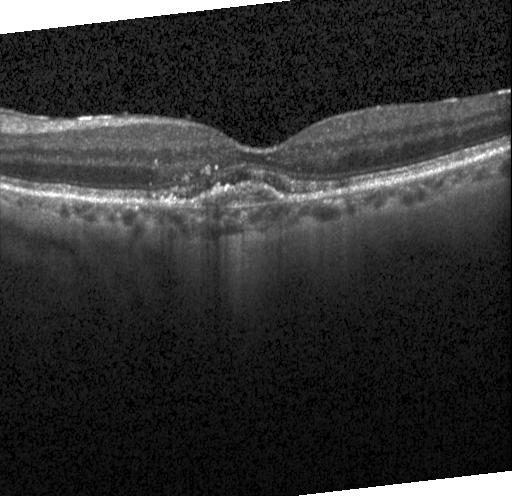 Centered on the fovea, SD-OCT, OCT B-scan
Impression: CNV.